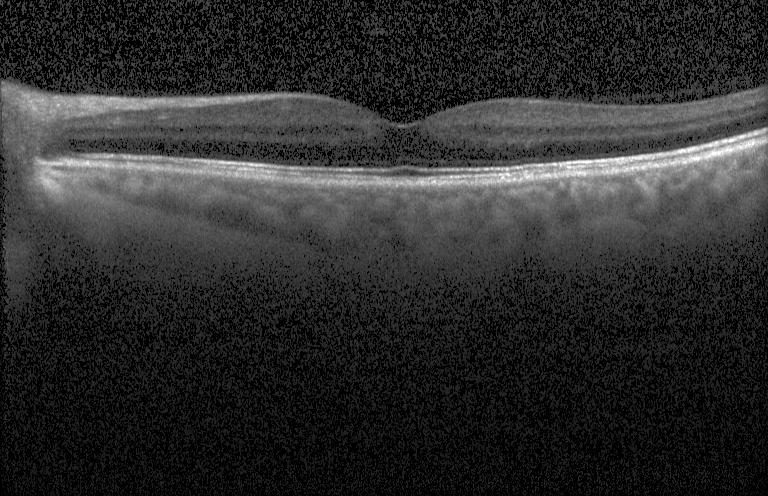 Optical coherence tomography B-scan.
Macular OCT: no choroidal neovascularization, no diabetic macular edema, and no drusen.